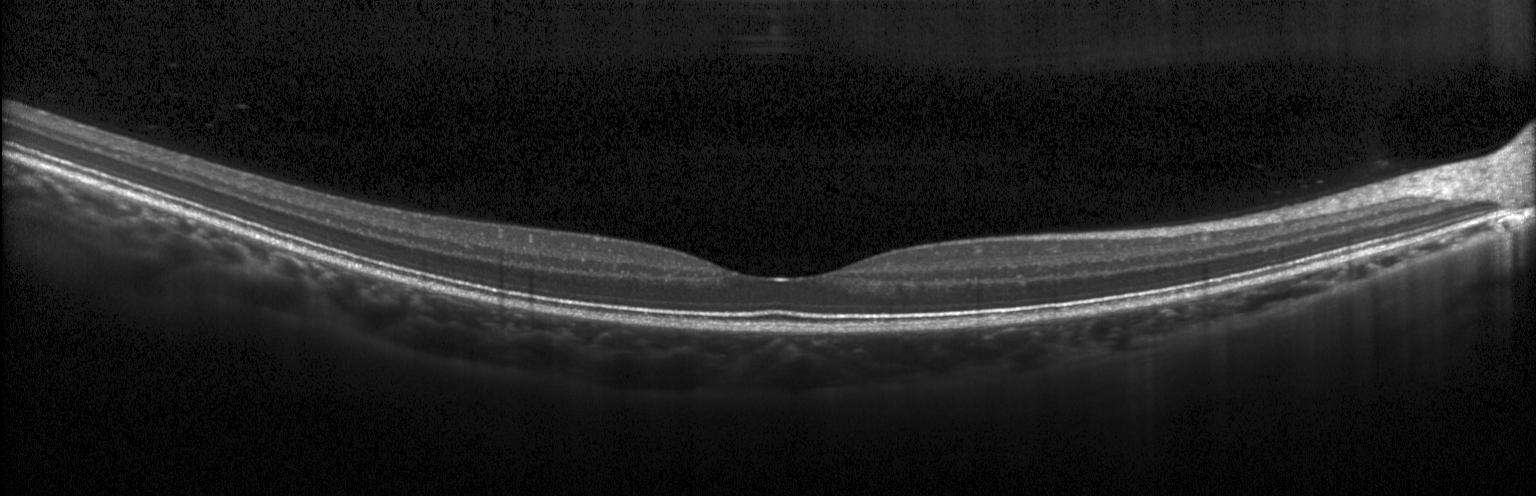
SD-OCT; fovea-centered; OCT B-scan — This B-scan demonstrates no choroidal neovascularization, no diabetic macular edema, and no drusen.